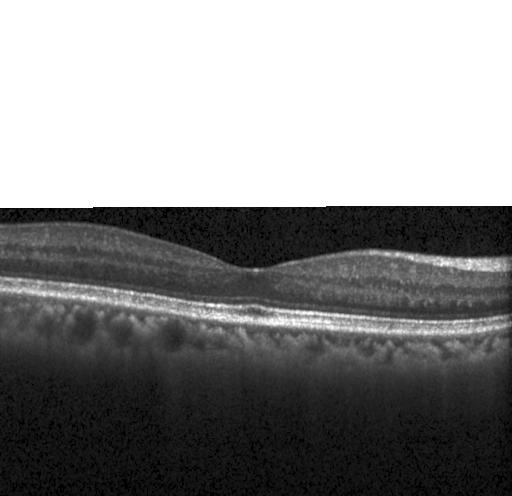 Optical coherence tomography B-scan, Heidelberg Spectralis, spectral-domain OCT
Macular OCT: no CNV, no DME, and no drusen.